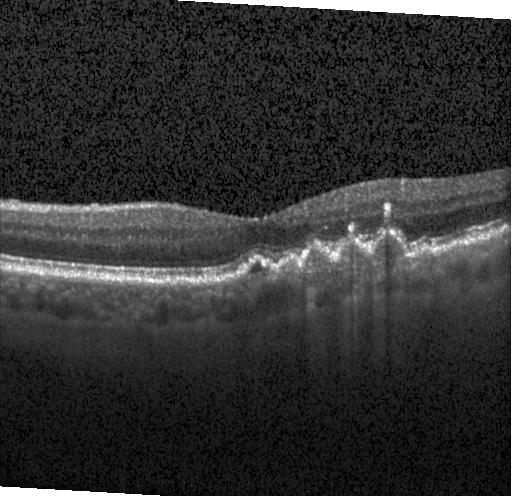

Macular scan; optical coherence tomography scan; spectral-domain optical coherence tomography; acquired on a Heidelberg Spectralis
The scan shows multiple drusen.